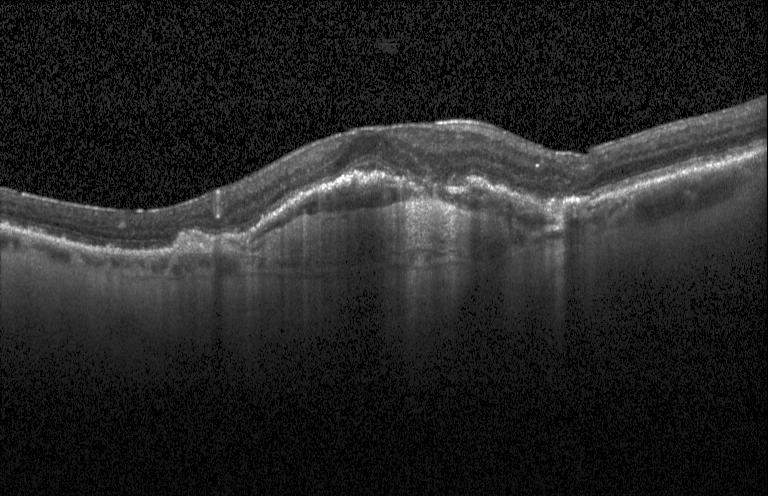
Spectral-domain optical coherence tomography, Heidelberg Spectralis OCT system, macular scan, retinal OCT cross-section
Impression: a choroidal neovascular membrane.